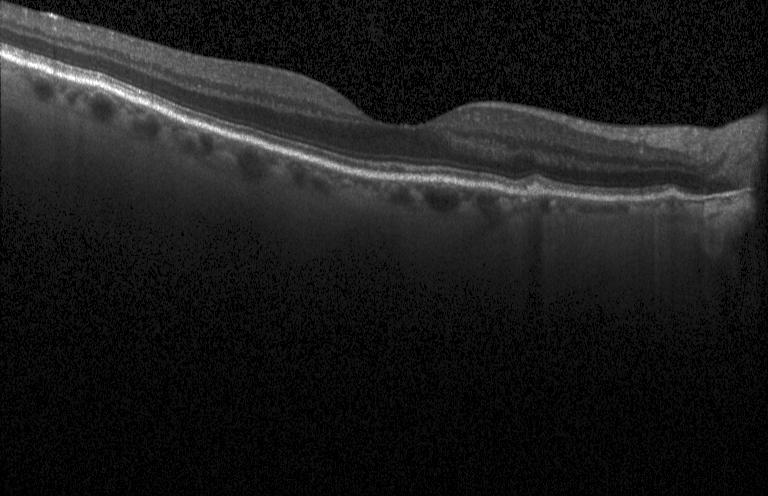

Drusen.